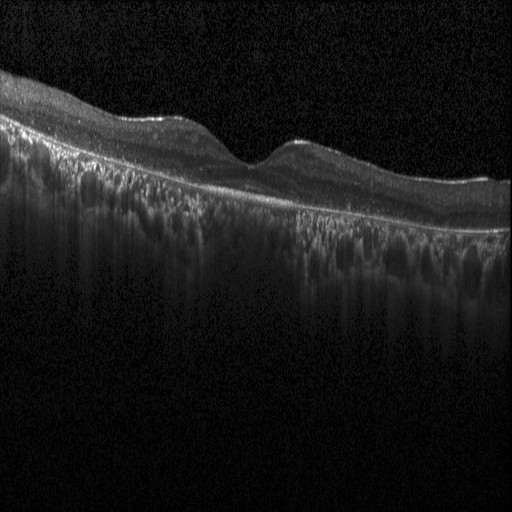 OCT B-scan showing DME.